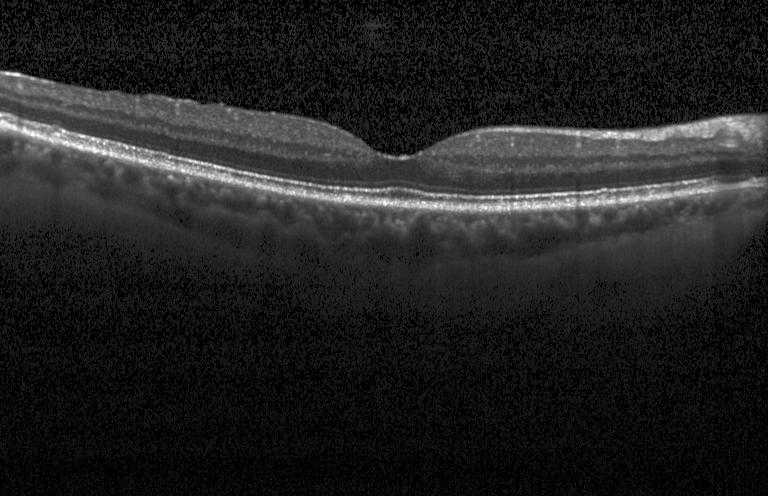
OCT line scan. Acquired on a Heidelberg Spectralis. Spectral-domain OCT. Macular scan — The scan shows no evidence of choroidal neovascularization, diabetic macular edema, or drusen.